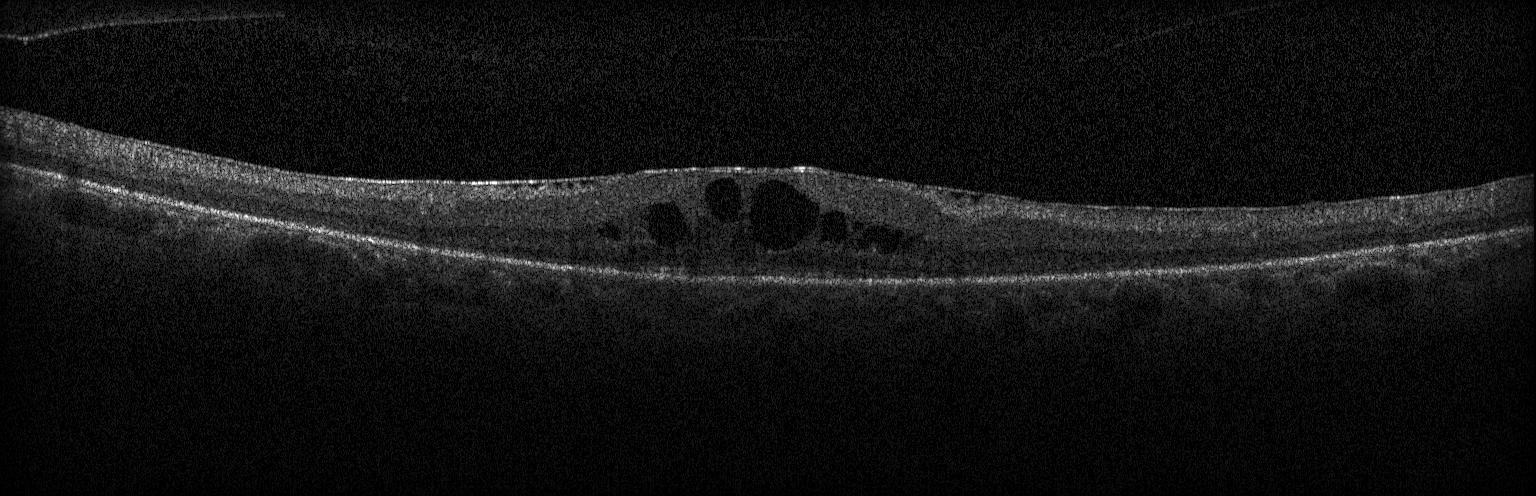
OCT scan showing diabetic macular edema.